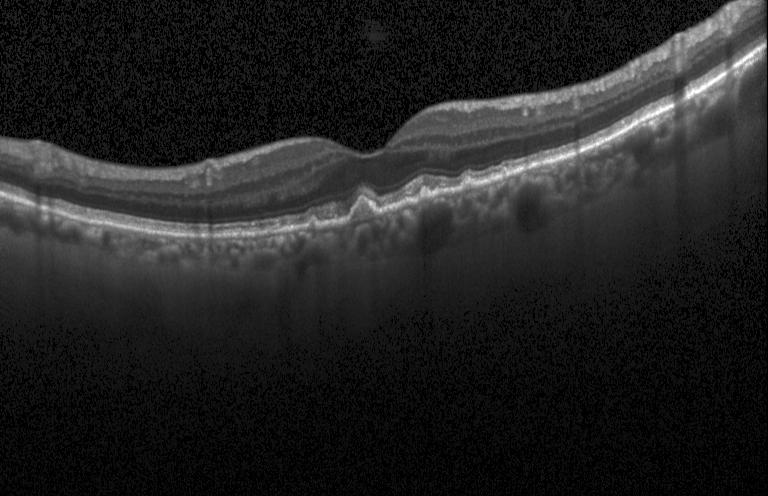

OCT B-scan — This B-scan demonstrates sub-RPE drusenoid deposits.